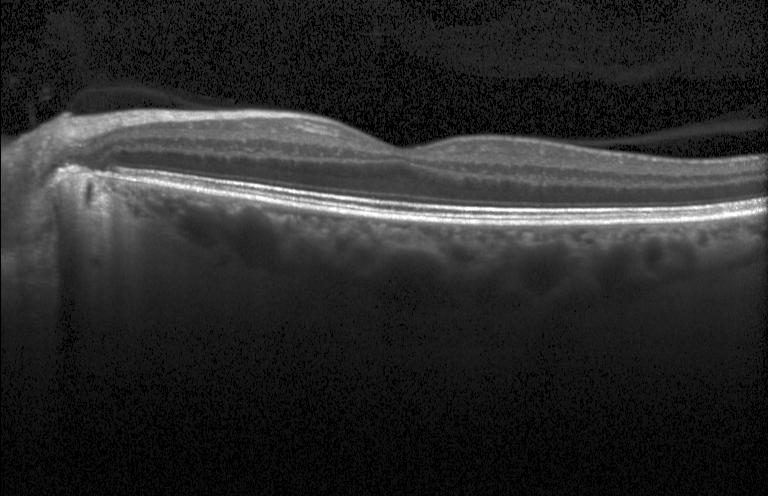

Optical coherence tomography scan — No choroidal neovascularization, no diabetic macular edema, and no drusen.